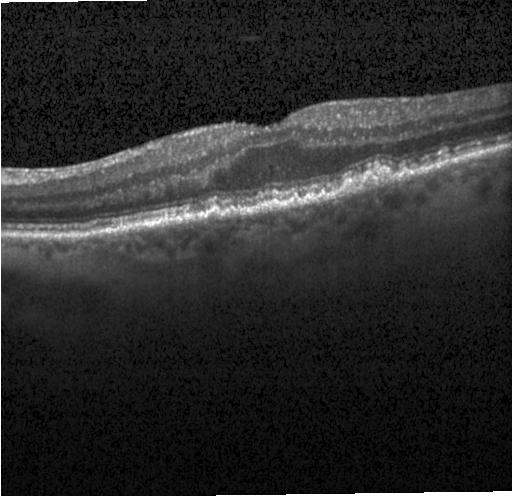
Instrument: Heidelberg Spectralis. OCT B-scan — Diagnosis: sub-RPE drusenoid deposits.